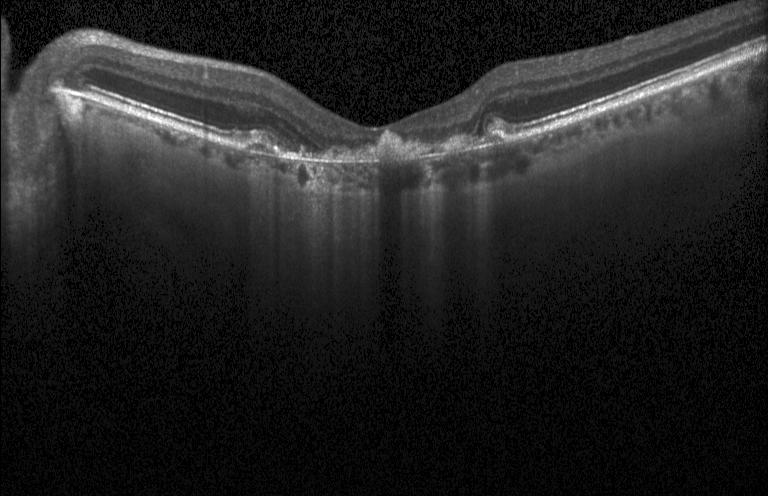 OCT B-scan showing choroidal neovascularization.